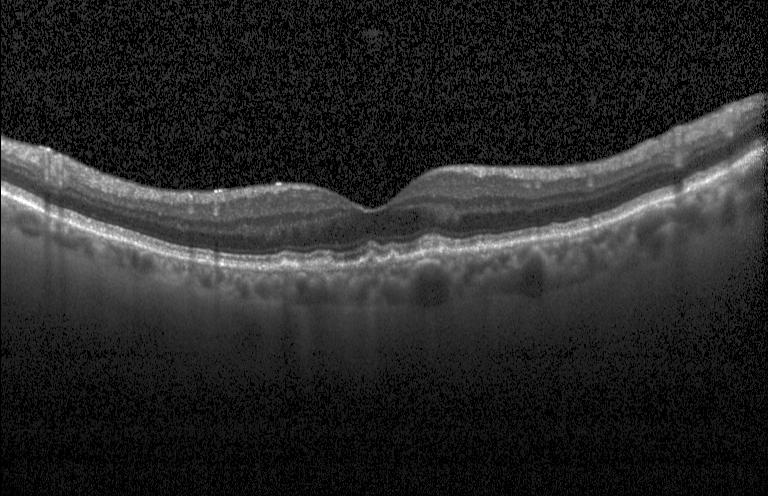

Heidelberg Spectralis · optical coherence tomography scan · SD-OCT.
Impression: drusen.